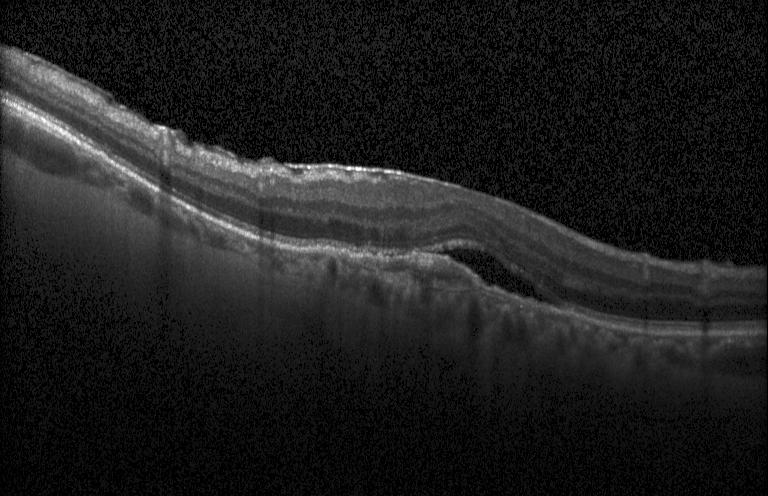

OCT line scan
The scan shows CNV.